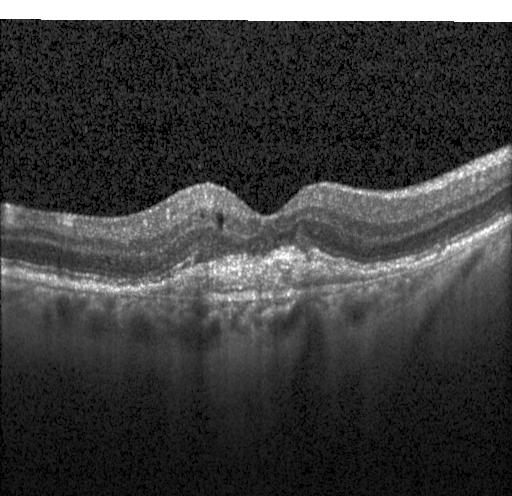 Through the macula, OCT line scan, spectral-domain optical coherence tomography
Finding: a choroidal neovascular membrane.